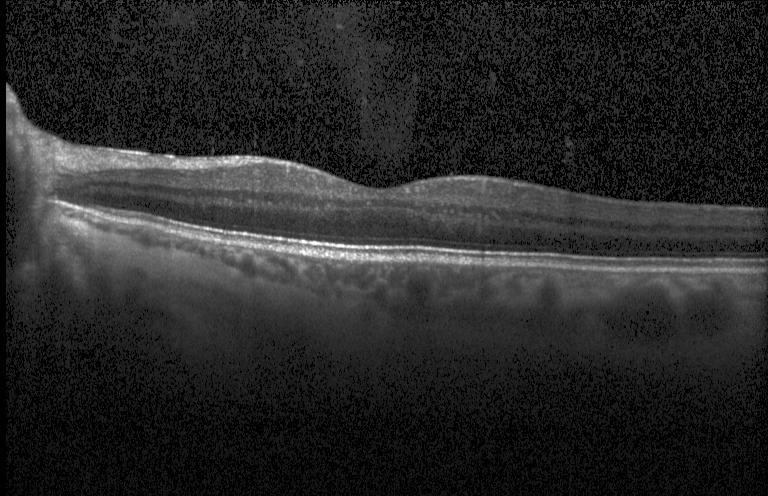 Macular OCT: neither CNV, DME, nor drusen.